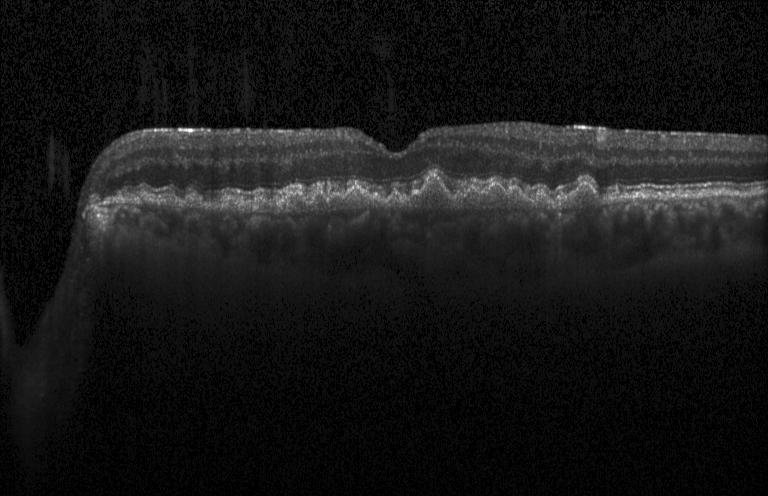
Spectral-domain OCT B-scan: a choroidal neovascular membrane.